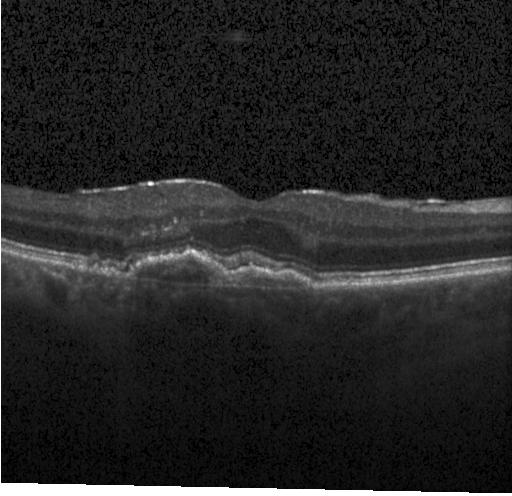 Macular OCT: choroidal neovascularization (CNV).